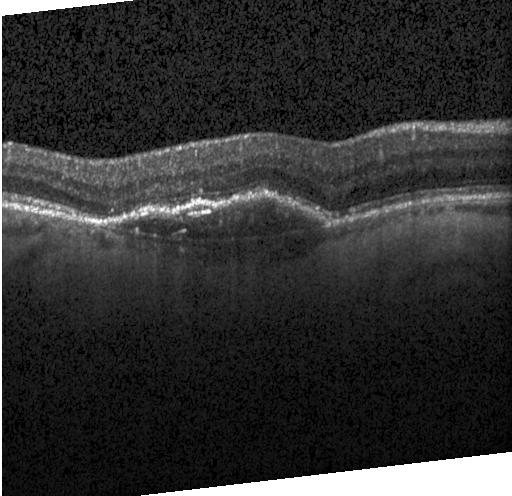
OCT line scan. Macular OCT: choroidal neovascularization (CNV).